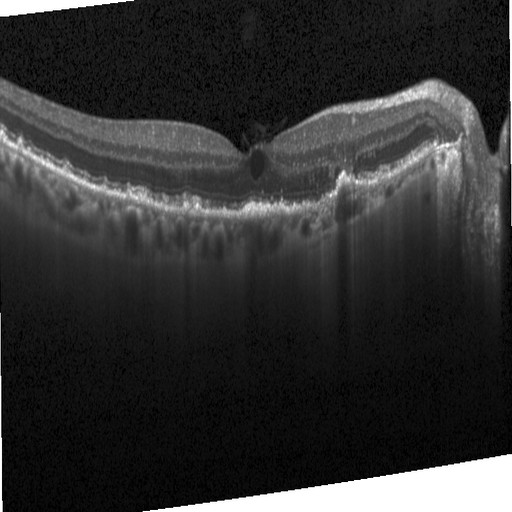 Finding: DME.